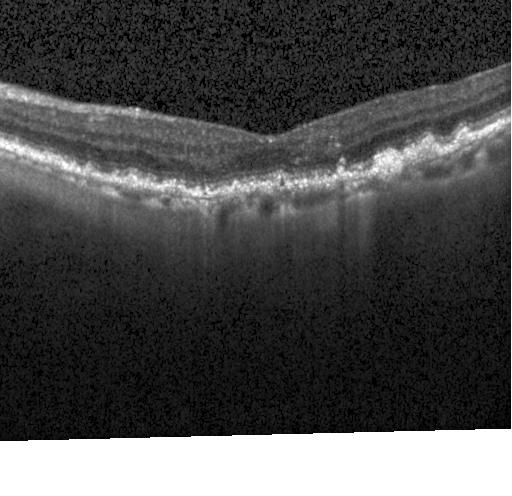

OCT B-scan — Impression: multiple drusen.